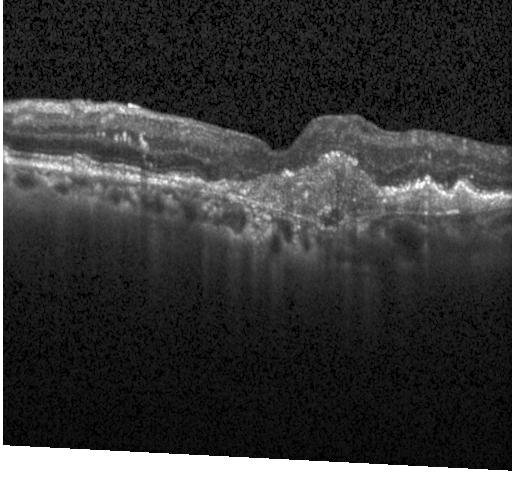

Optical coherence tomography B-scan, Heidelberg Spectralis OCT system. Impression: CNV.